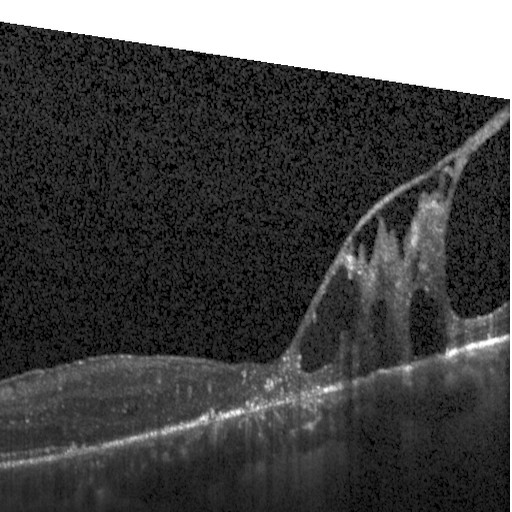

Retinal OCT cross-section showing DME.